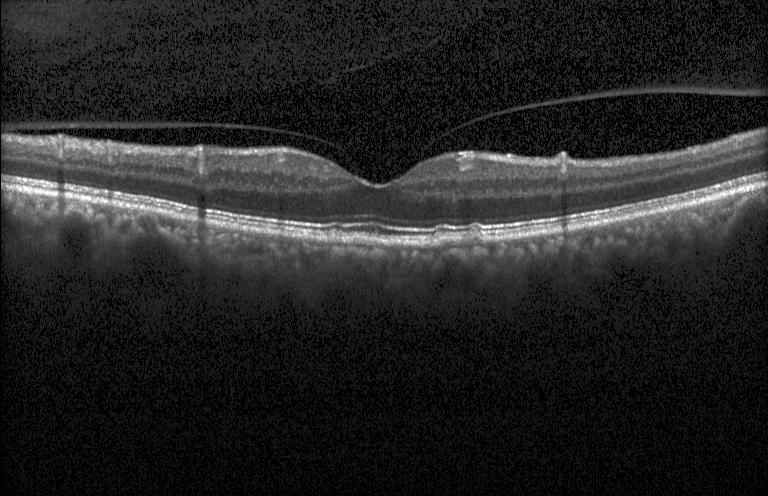

Impression: sub-RPE drusenoid deposits.